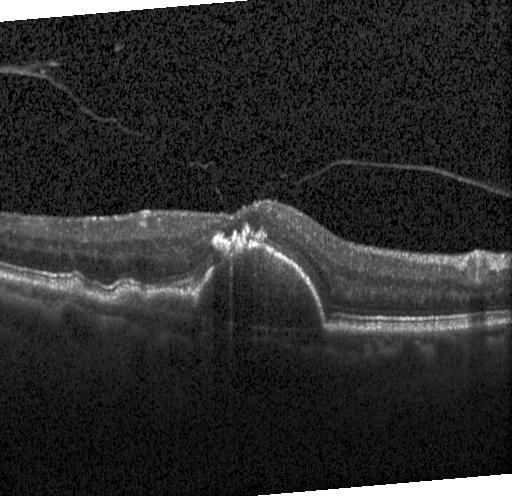

Optical coherence tomography scan. Diagnosis: choroidal neovascularization (CNV).